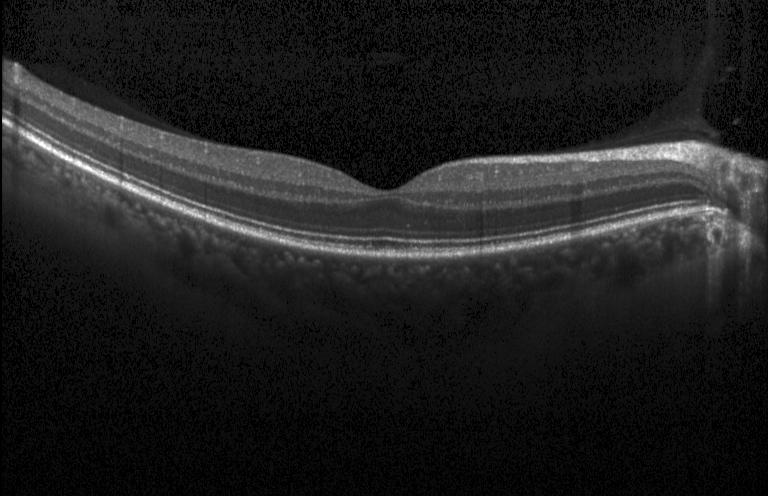 Optical coherence tomography B-scan; spectral-domain OCT
Impression: no evidence of choroidal neovascularization, diabetic macular edema, or drusen.